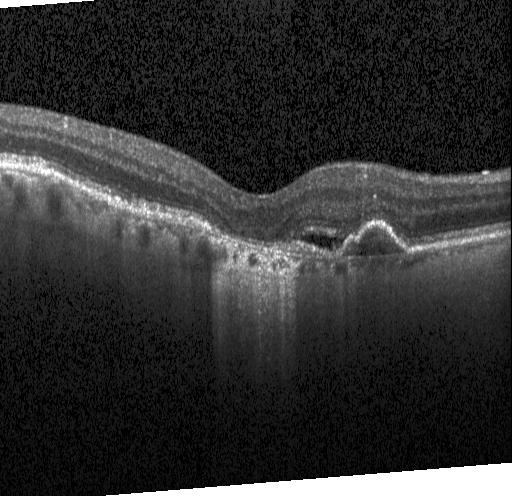

Macular OCT: a choroidal neovascular membrane.